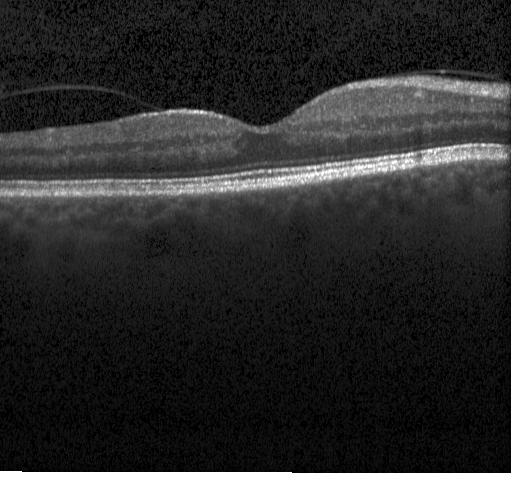

Heidelberg Spectralis OCT system, optical coherence tomography scan, centered on the fovea
Impression: no choroidal neovascularization, diabetic macular edema, or drusen.